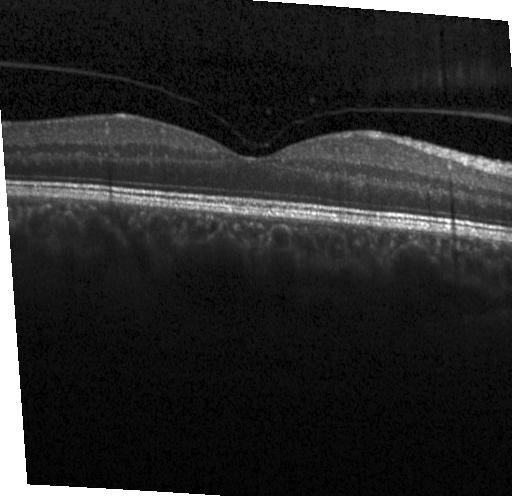 Impression: neither choroidal neovascularization, diabetic macular edema, nor drusen.